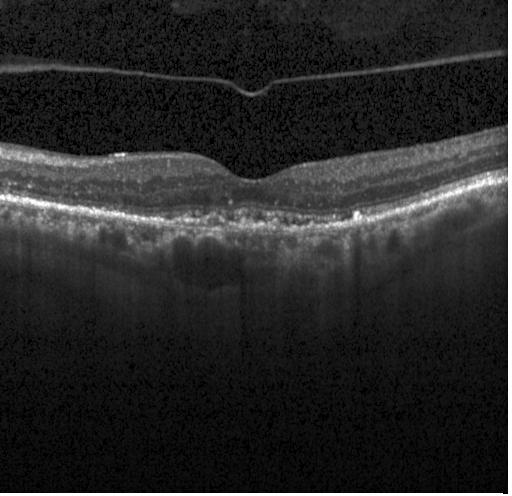 Optical coherence tomography B-scan. Spectral-domain optical coherence tomography. Heidelberg Spectralis OCT system
Impression: choroidal neovascularization.